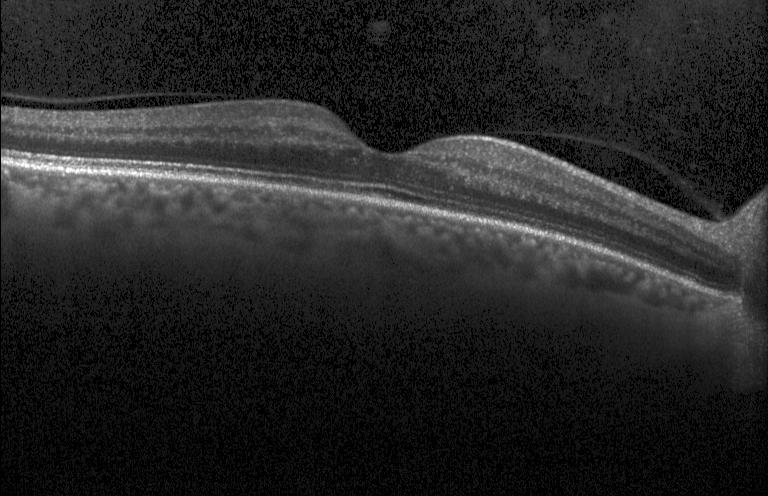 Acquired on a Heidelberg Spectralis. Optical coherence tomography scan. Spectral-domain OCT.
Finding: no evidence of choroidal neovascularization, diabetic macular edema, or drusen.